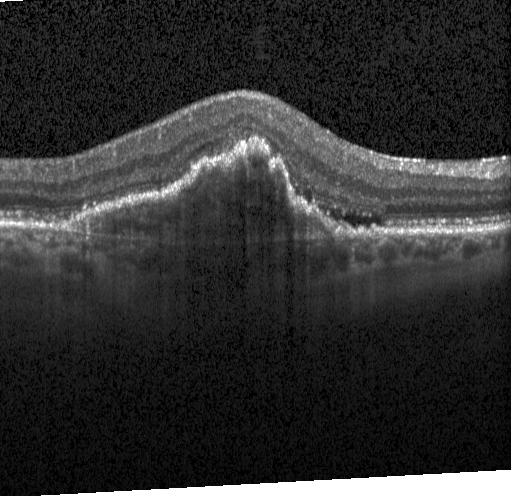
Dx: CNV.